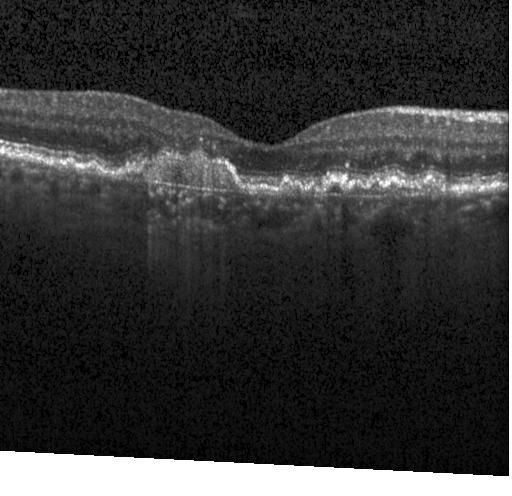 Diagnosis: choroidal neovascularization.